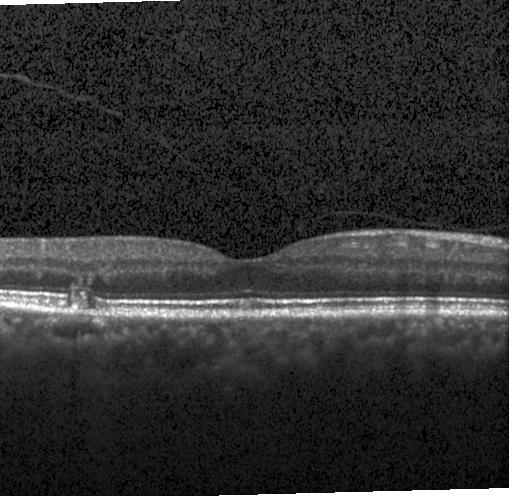
Optical coherence tomography B-scan — No evidence of CNV, DME, or drusen.